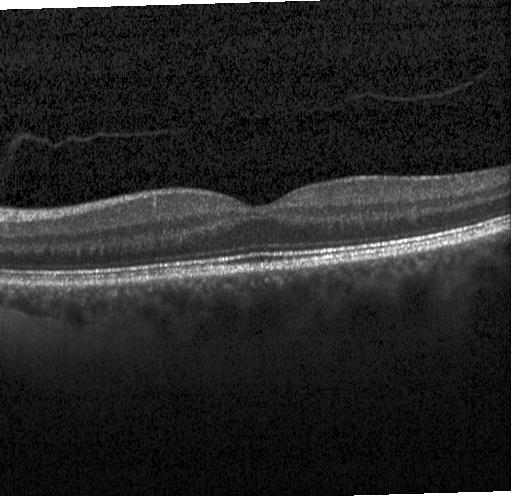 OCT B-scan; instrument: Heidelberg Spectralis.
OCT finding: no evidence of CNV, DME, or drusen.